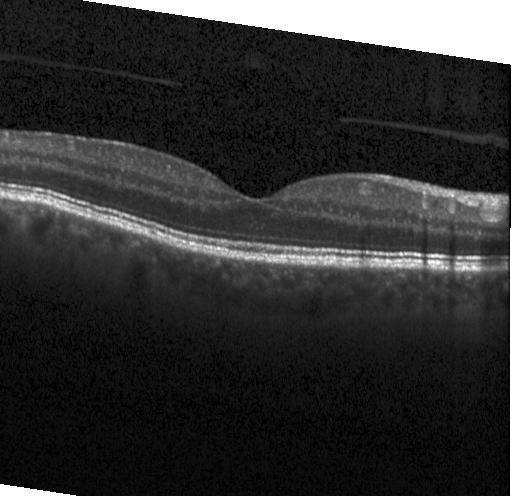
Impression: no CNV, no DME, and no drusen.